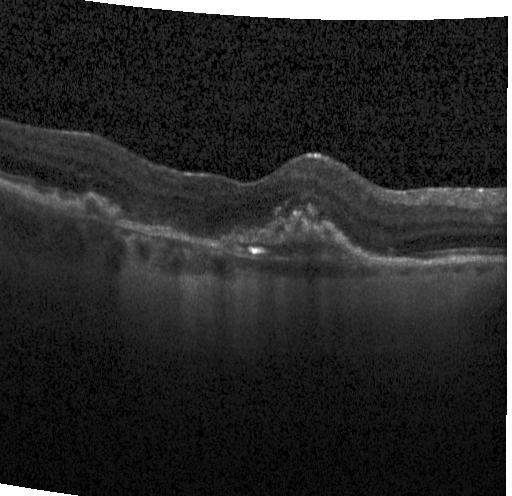 Spectral-domain OCT B-scan: choroidal neovascularization (CNV).